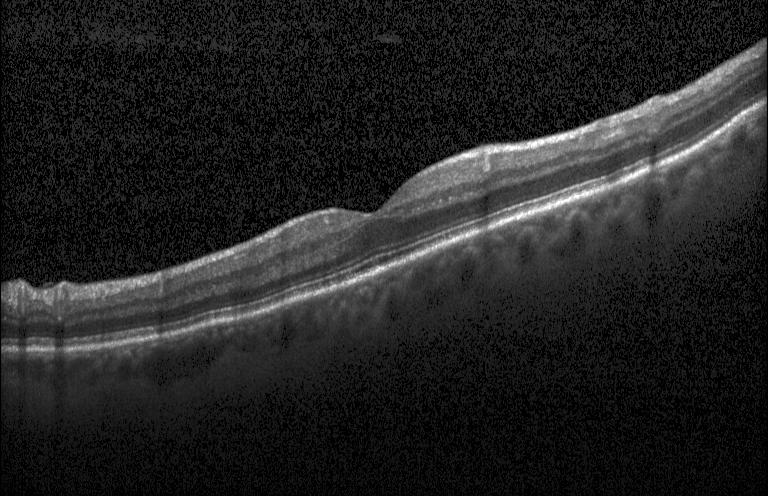
Centered on the fovea. Acquired on a Heidelberg Spectralis. OCT B-scan
OCT finding: no CNV, DME, or drusen.